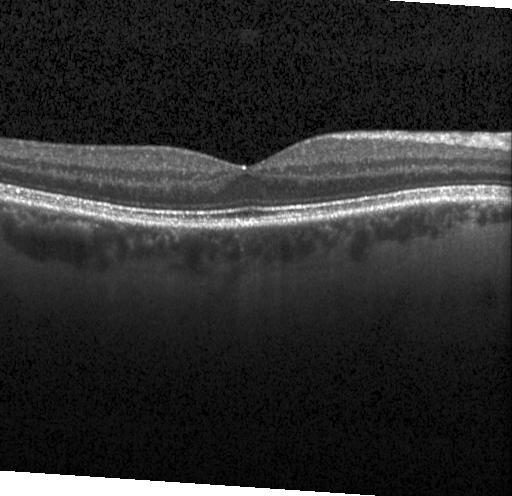

OCT B-scan showing no choroidal neovascularization, diabetic macular edema, or drusen.